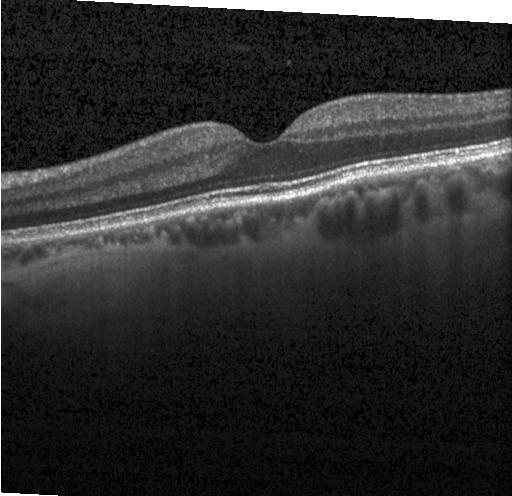

Optical coherence tomography scan, spectral-domain OCT, acquired on a Heidelberg Spectralis
Assessment: no evidence of choroidal neovascularization, diabetic macular edema, or drusen.